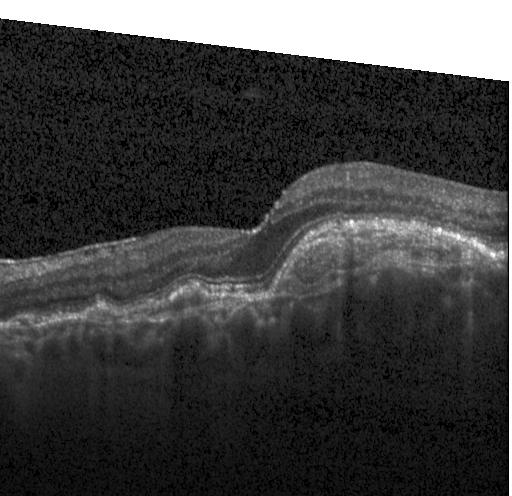 Macular scan, optical coherence tomography B-scan, instrument: Heidelberg Spectralis — Diagnosis: choroidal neovascularization (CNV).